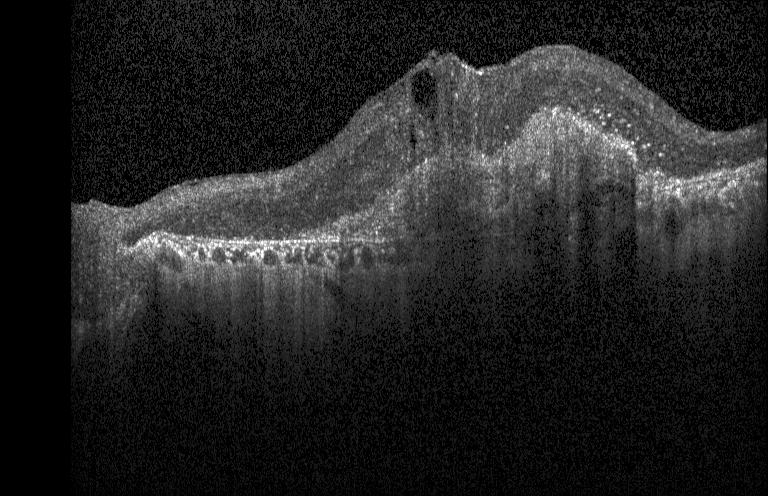

Through the macula; Heidelberg Spectralis OCT system; SD-OCT; optical coherence tomography scan
Dx: a choroidal neovascular membrane.